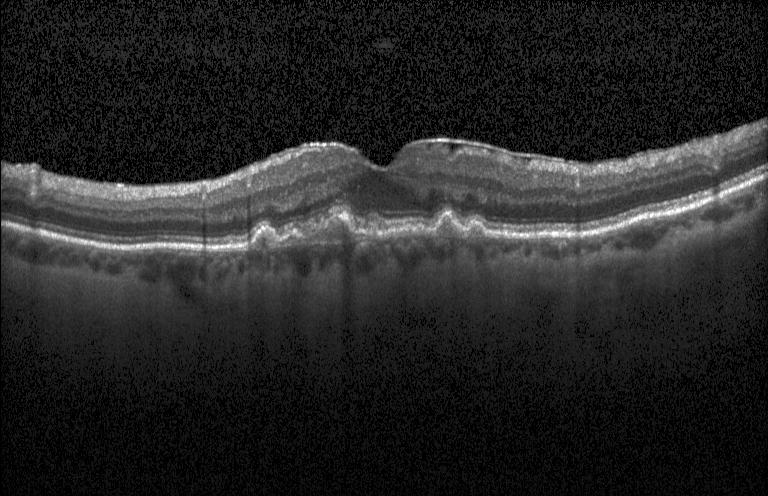
OCT B-scan — Sub-RPE drusenoid deposits.